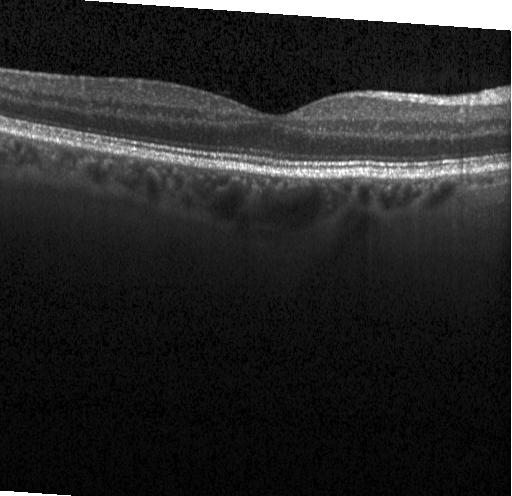
SD-OCT. Optical coherence tomography B-scan — This B-scan demonstrates no CNV, DME, or drusen.